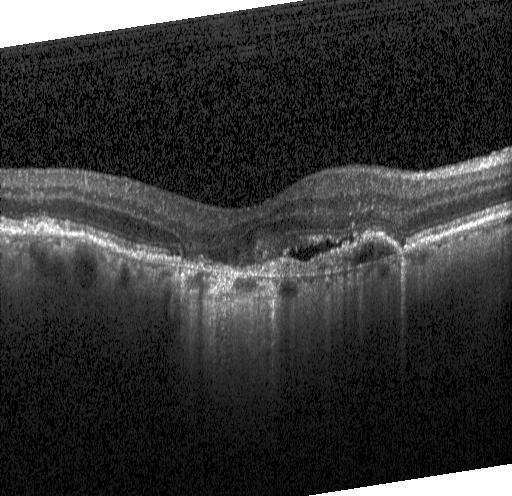

Spectral-domain optical coherence tomography. Fovea-centered. Heidelberg Spectralis OCT system. Optical coherence tomography B-scan. Finding: choroidal neovascularization (CNV).